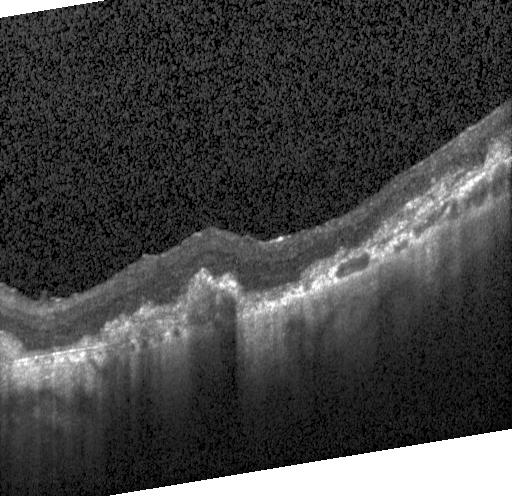
Optical coherence tomography B-scan, centered on the fovea, Heidelberg Spectralis. Finding: a choroidal neovascular membrane.